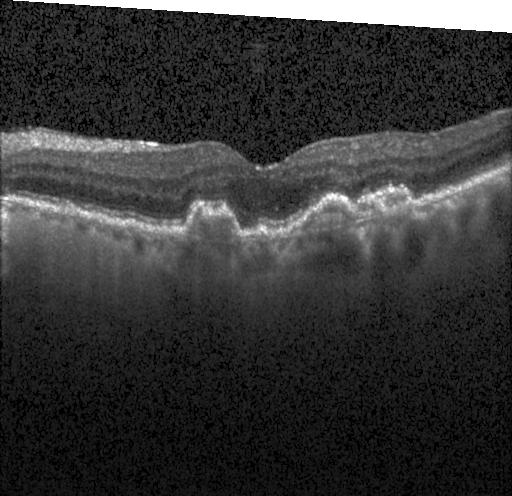
Through the macula, OCT B-scan
Assessment: choroidal neovascularization (CNV).